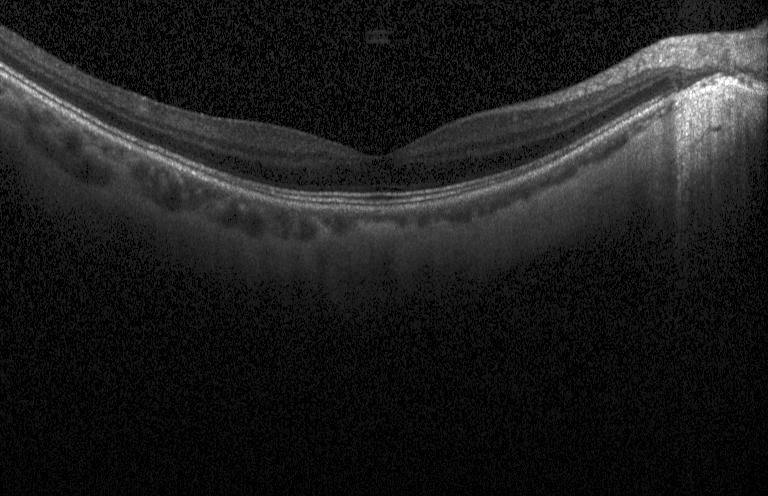 Macular OCT: no CNV, DME, or drusen.